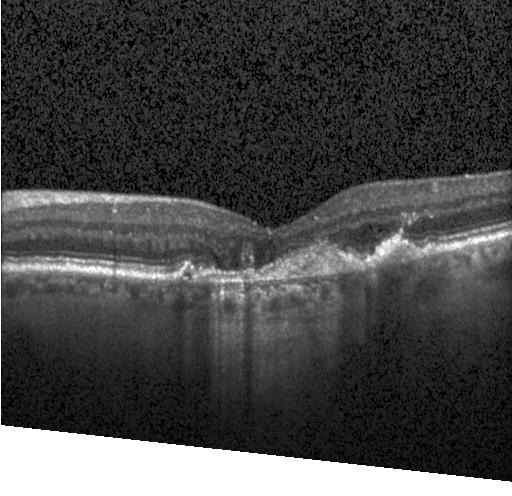
Through the macula · spectral-domain optical coherence tomography · instrument: Heidelberg Spectralis · optical coherence tomography scan
Macular OCT: a choroidal neovascular membrane.